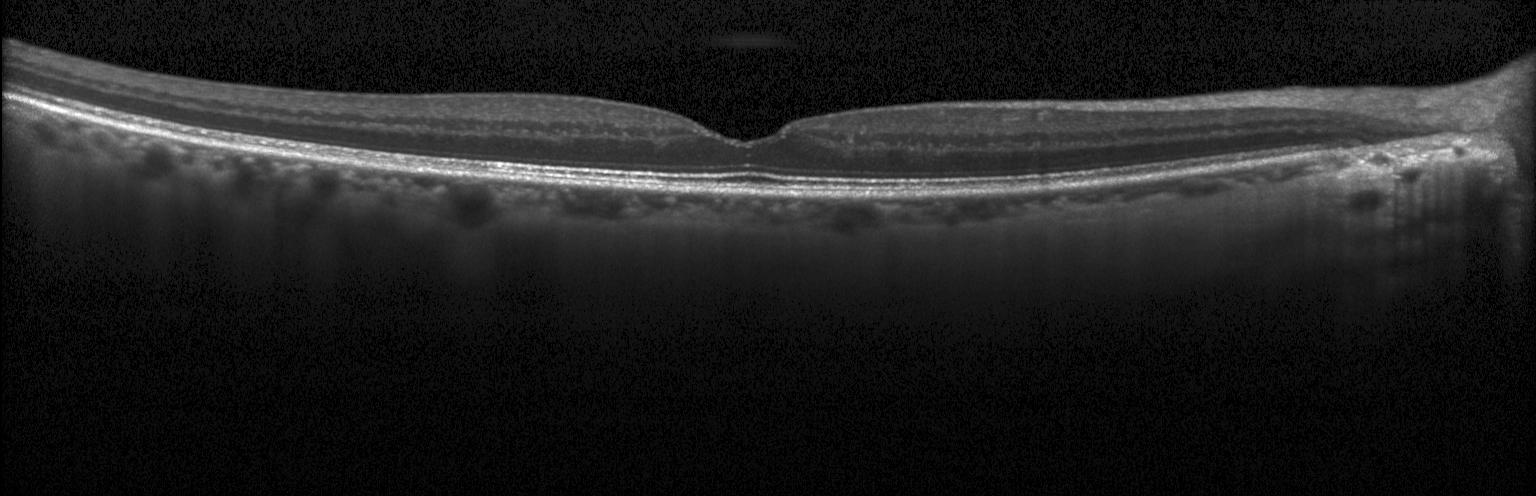 Macular OCT: neither choroidal neovascularization, diabetic macular edema, nor drusen.